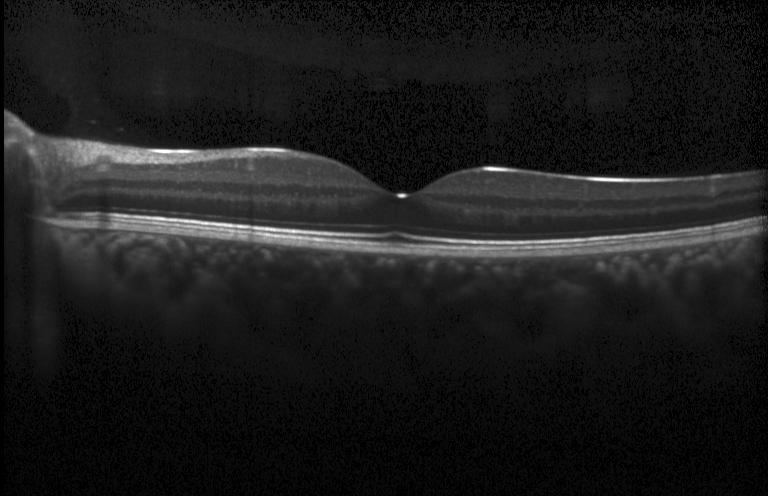

Optical coherence tomography B-scan. Fovea-centered. Heidelberg Spectralis OCT system.
Diagnosis: no choroidal neovascularization, diabetic macular edema, or drusen.